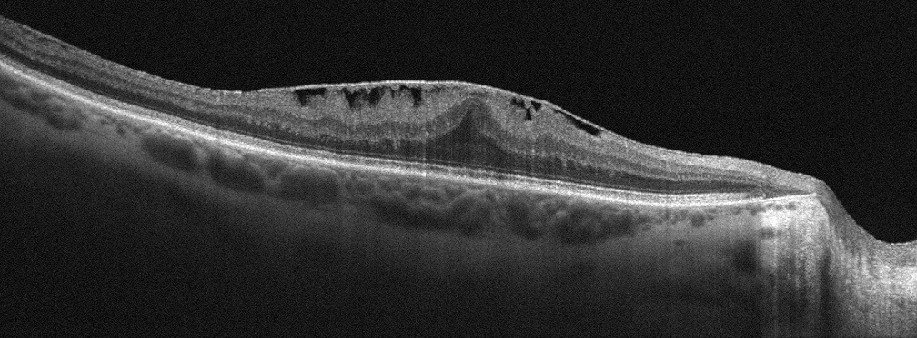
Dx: epiretinal membrane (ERM).